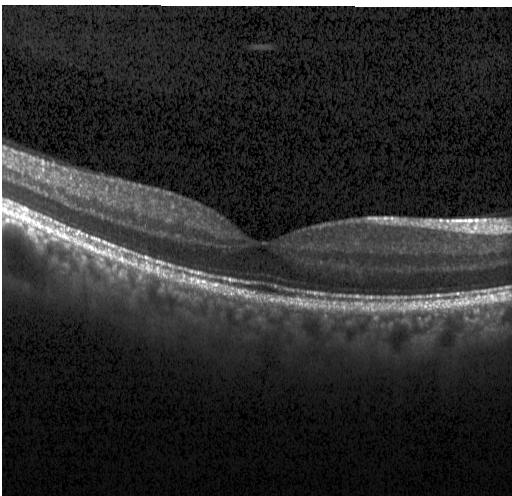
Instrument: Heidelberg Spectralis, SD-OCT, optical coherence tomography scan — Impression: no evidence of CNV, DME, or drusen.